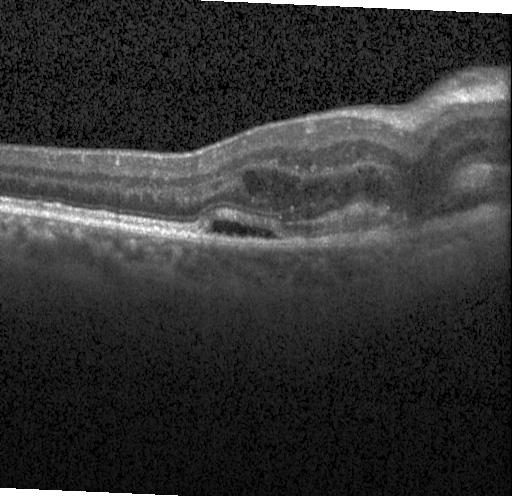

Spectral-domain OCT B-scan: a choroidal neovascular membrane.